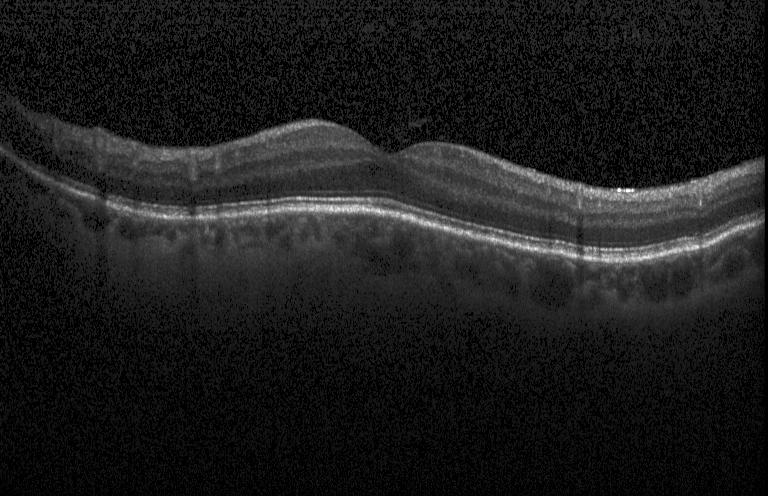
Retinal OCT cross-section
Finding: no CNV, DME, or drusen.